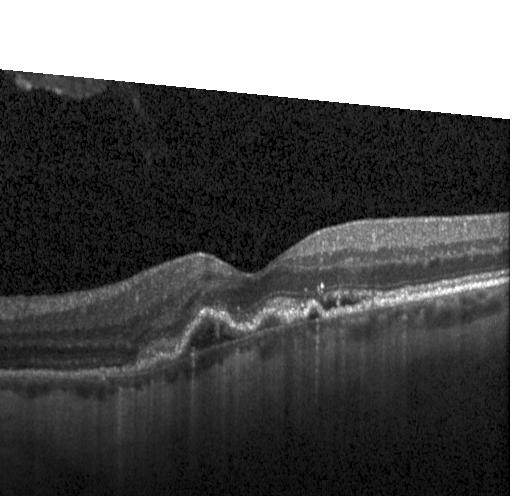 Spectral-domain OCT · retinal OCT B-scan. This B-scan demonstrates choroidal neovascularization.